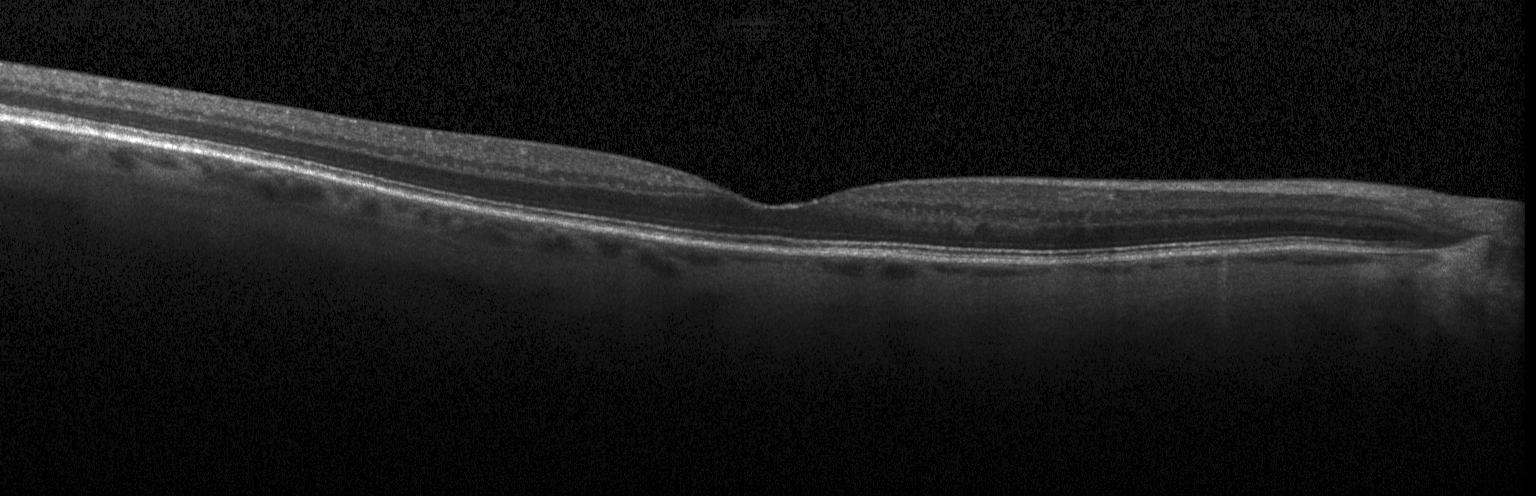

Horizontal scan through the fovea, spectral-domain optical coherence tomography, optical coherence tomography scan, Heidelberg Spectralis
OCT finding: no choroidal neovascularization, no diabetic macular edema, and no drusen.